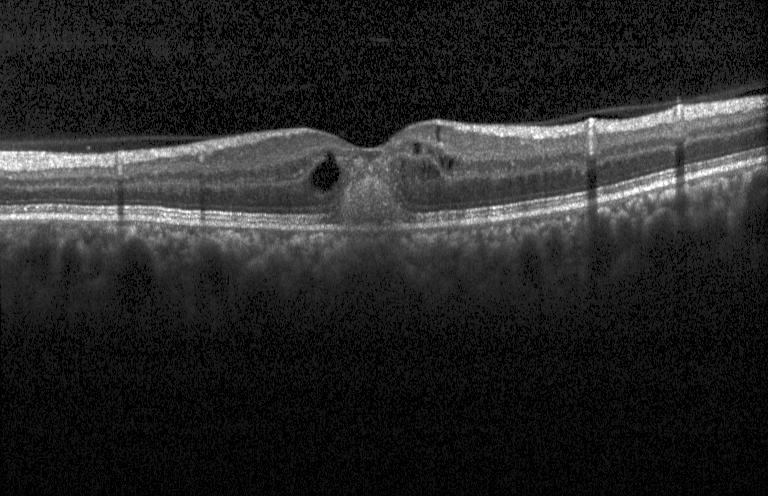 Dx: a choroidal neovascular membrane.